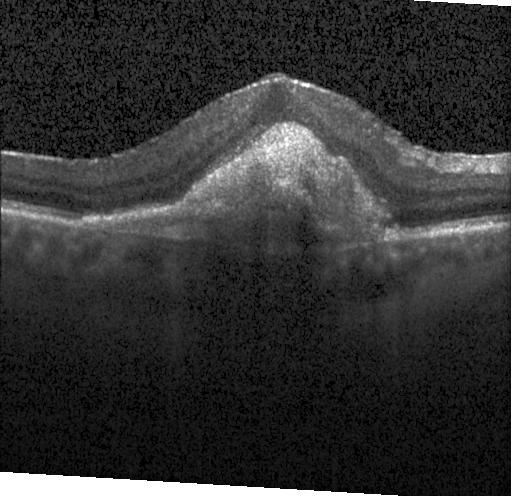 OCT finding: a choroidal neovascular membrane.